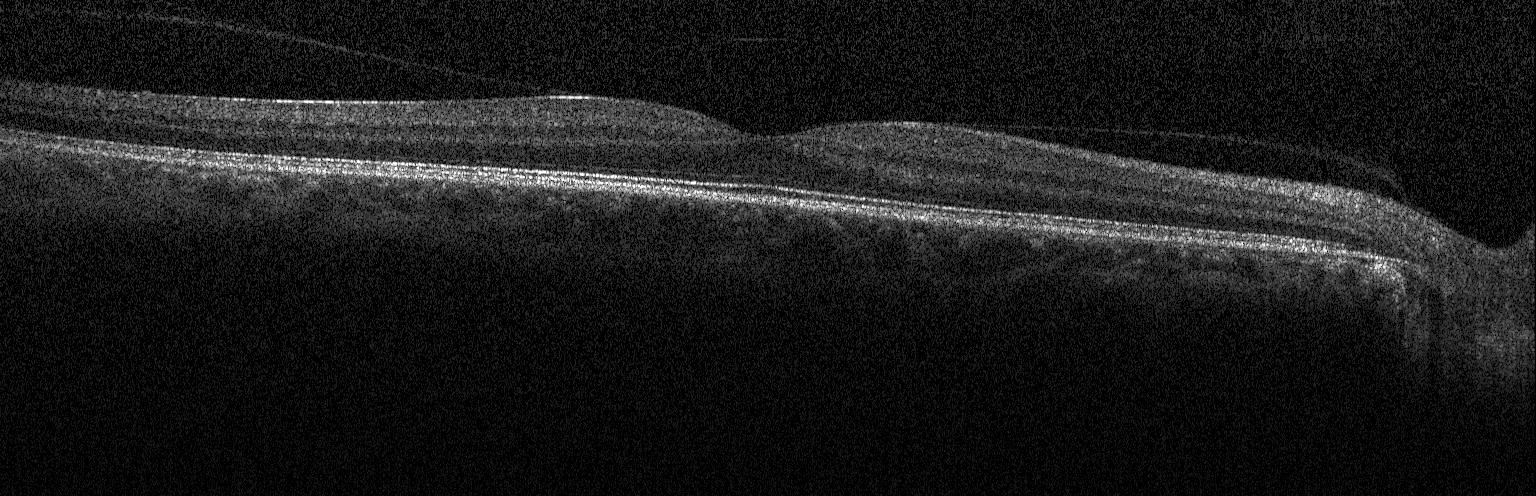 Macular OCT: no choroidal neovascularization, no diabetic macular edema, and no drusen.